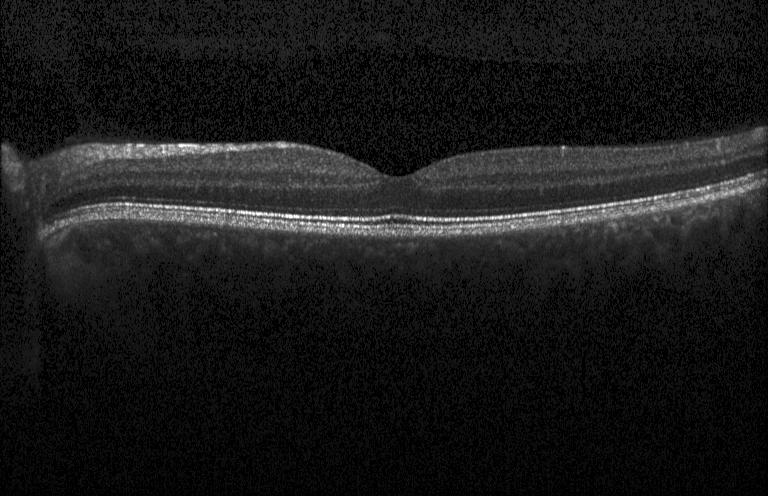 Impression: no evidence of choroidal neovascularization, diabetic macular edema, or drusen.